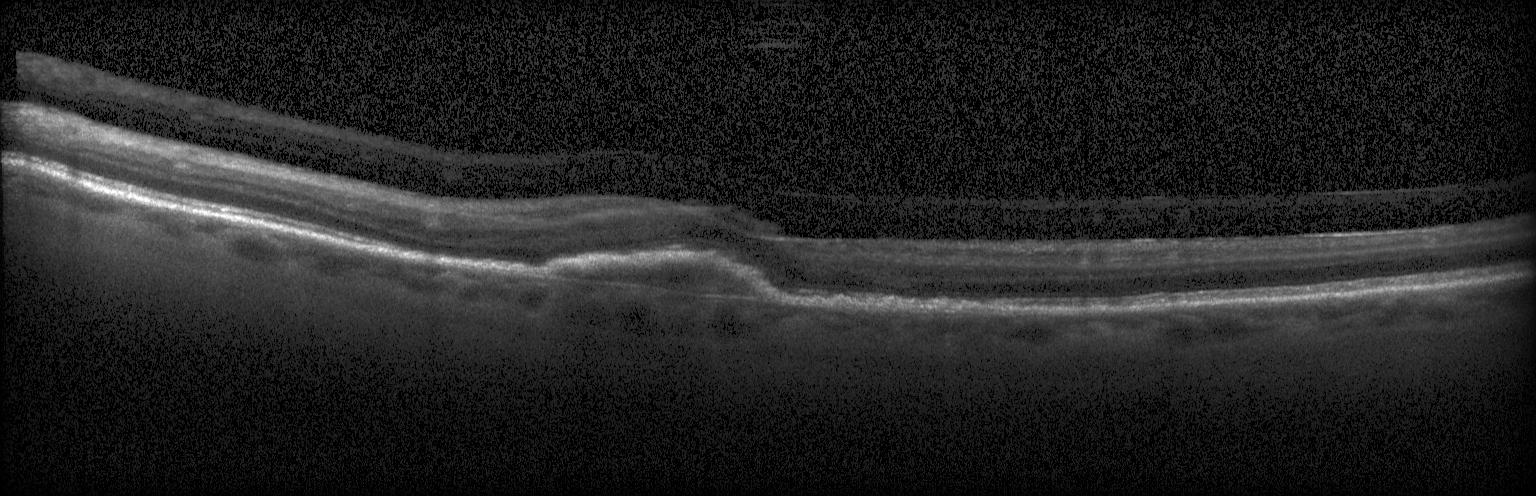

Macular scan · OCT line scan · Heidelberg Spectralis OCT system · spectral-domain OCT. Diagnosis: choroidal neovascularization (CNV).